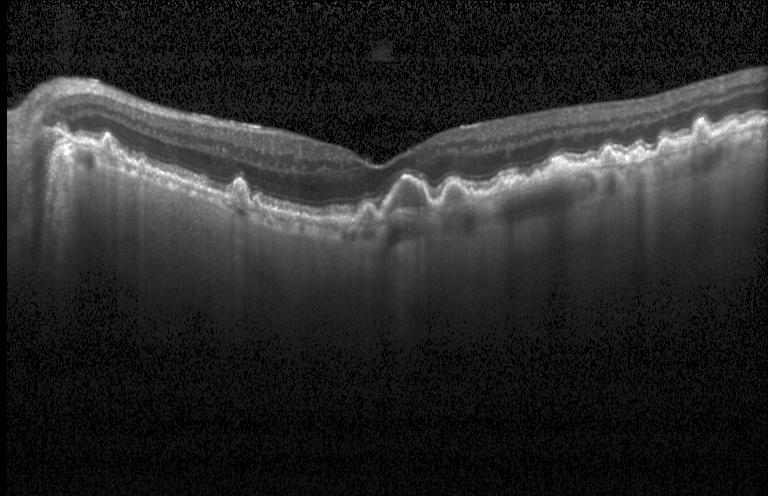 Fovea-centered. Spectral-domain optical coherence tomography. OCT line scan — The scan shows drusen.